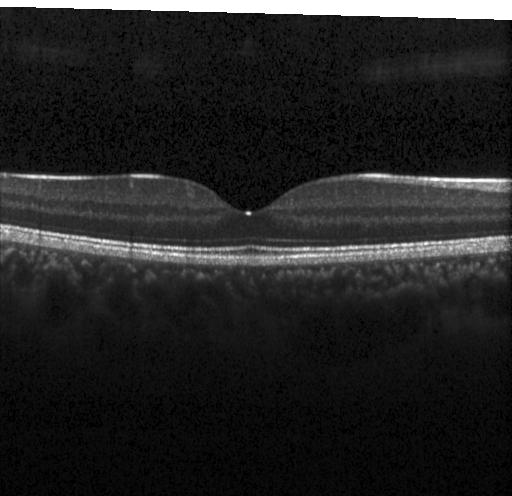
Dx: no CNV, no DME, and no drusen.